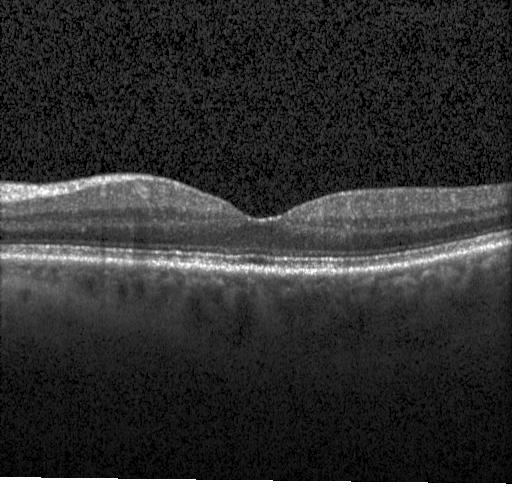 Impression: no evidence of choroidal neovascularization, diabetic macular edema, or drusen.